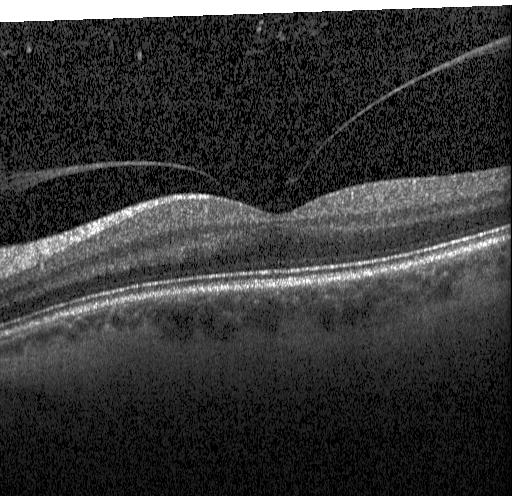
Macular OCT: no CNV, DME, or drusen.